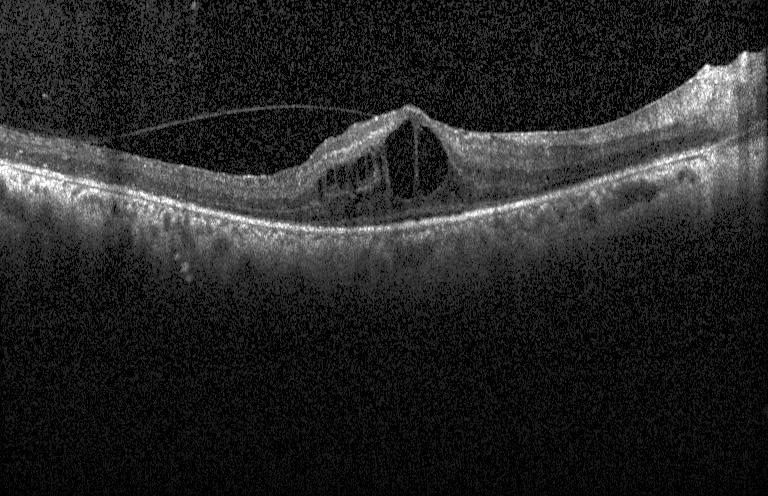 Retinal OCT B-scan. SD-OCT. Horizontal scan through the fovea.
OCT finding: DME.